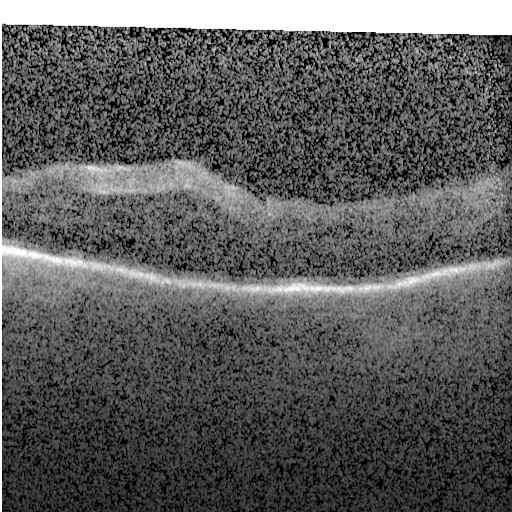

Retinal OCT cross-section, fovea-centered
Dx: DME.